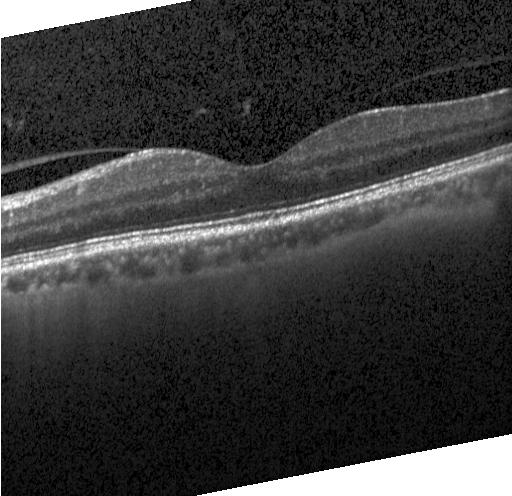

Assessment: no CNV, DME, or drusen.